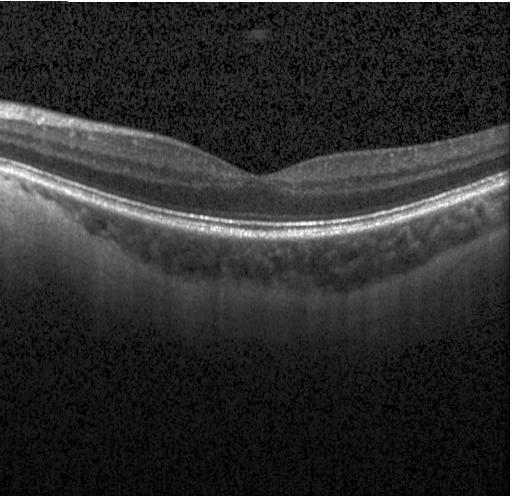

Heidelberg Spectralis OCT system. OCT B-scan.
This B-scan demonstrates no evidence of choroidal neovascularization, diabetic macular edema, or drusen.